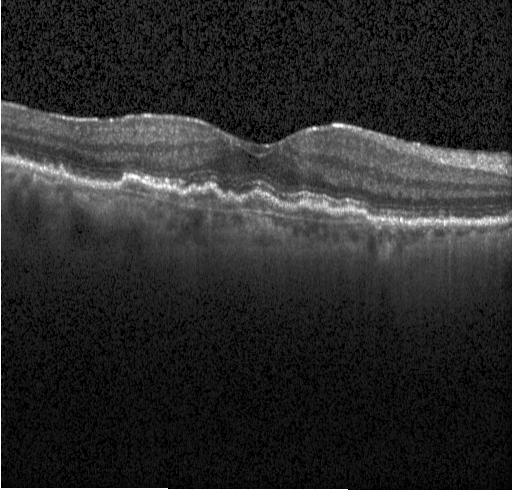
Instrument: Heidelberg Spectralis · optical coherence tomography B-scan · macular scan — Diagnosis: CNV.